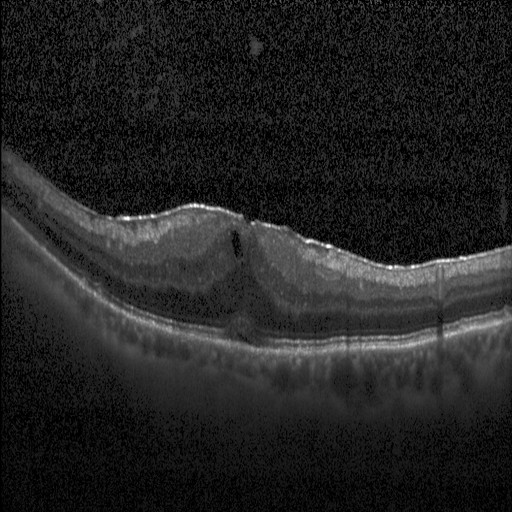

Centered on the fovea, spectral-domain optical coherence tomography, retinal OCT cross-section.
Finding: diabetic macular edema (DME).